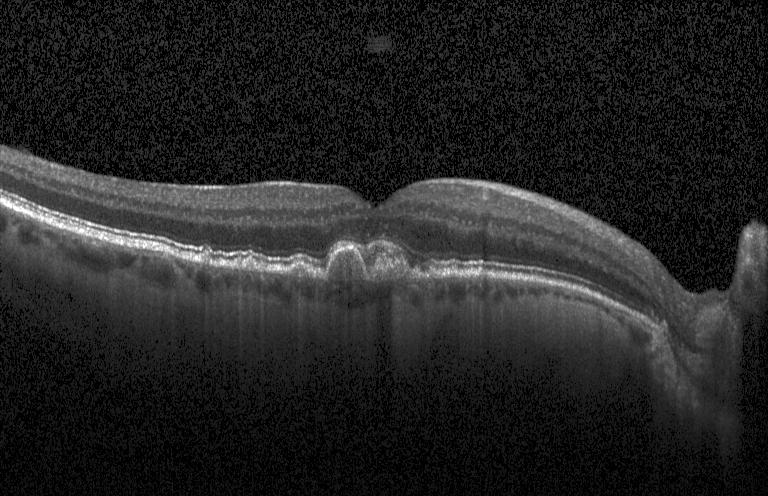
Heidelberg Spectralis · spectral-domain OCT · retinal OCT cross-section — Impression: multiple drusen.